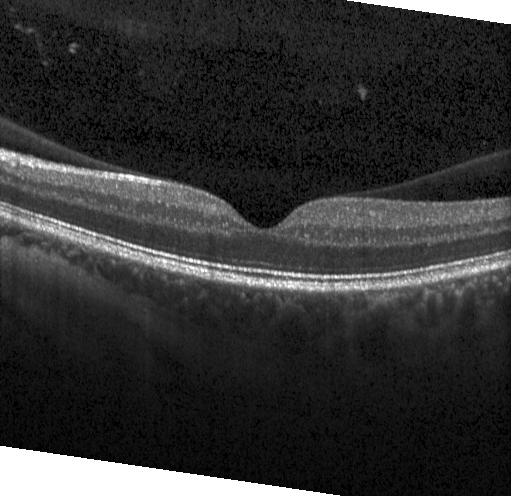
OCT B-scan showing neither CNV, DME, nor drusen.